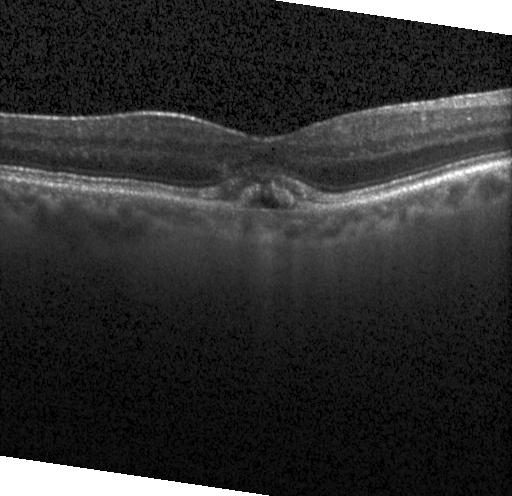
Optical coherence tomography B-scan. SD-OCT
OCT finding: a choroidal neovascular membrane.